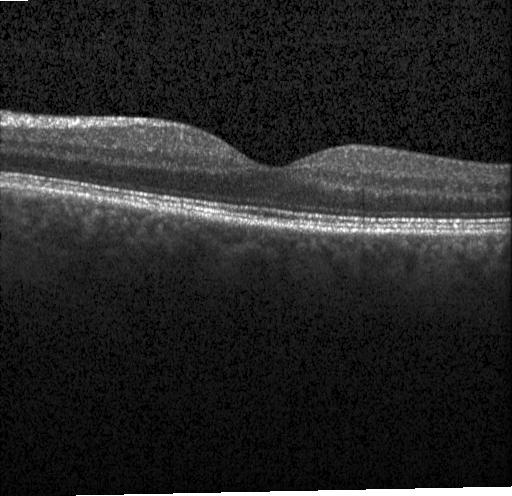 Through the macula. Heidelberg Spectralis OCT system. Optical coherence tomography scan. Dx: no choroidal neovascularization, no diabetic macular edema, and no drusen.